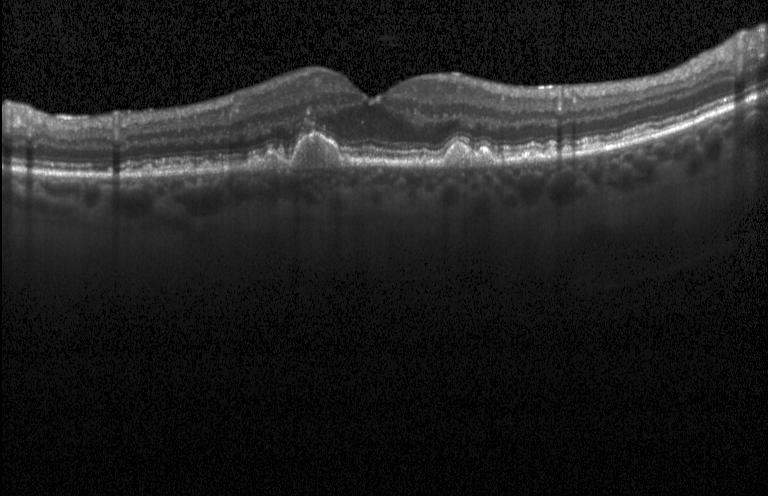

Optical coherence tomography scan. Dx: sub-RPE drusenoid deposits.